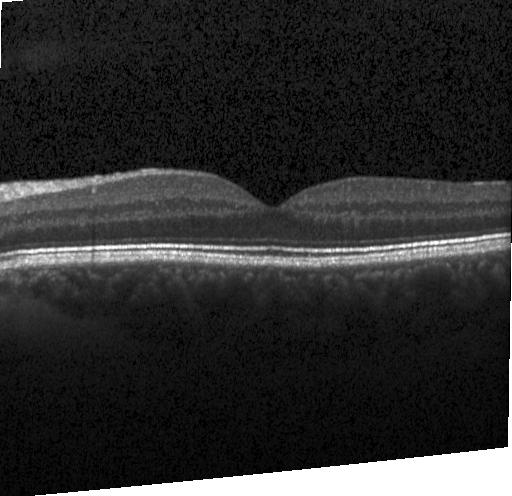

OCT line scan
This B-scan demonstrates no choroidal neovascularization, no diabetic macular edema, and no drusen.